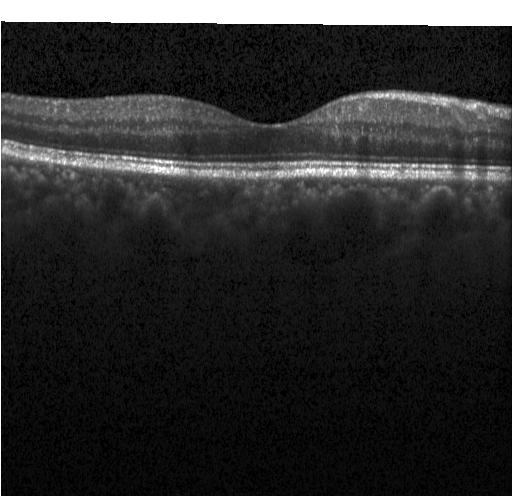
Acquired on a Heidelberg Spectralis · retinal OCT cross-section · through the macula · SD-OCT — Diagnosis: no evidence of CNV, DME, or drusen.